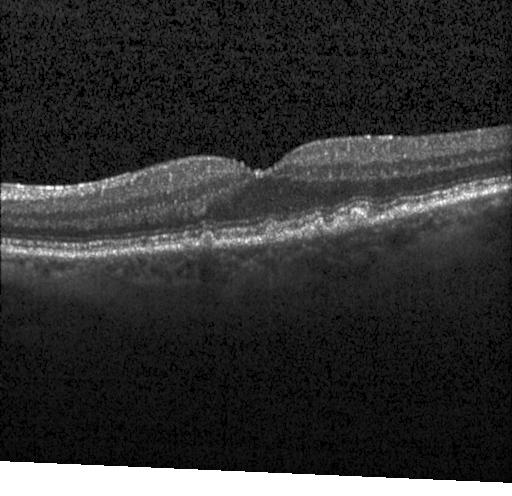 Optical coherence tomography scan · spectral-domain optical coherence tomography · Heidelberg Spectralis · macular scan — Macular OCT: sub-RPE drusenoid deposits.